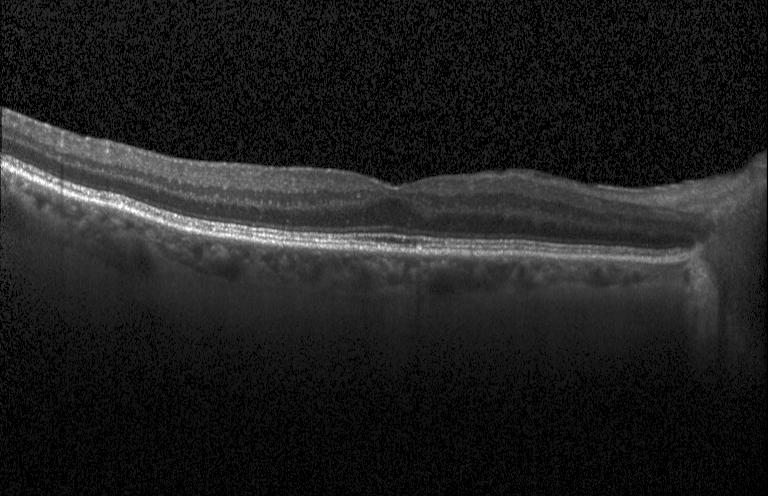
Dx: neither choroidal neovascularization, diabetic macular edema, nor drusen.